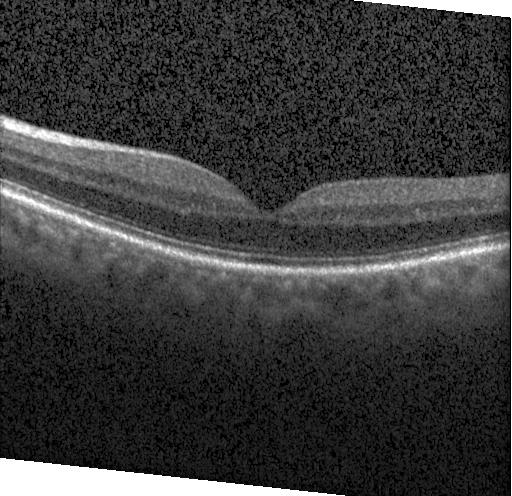
OCT line scan. Heidelberg Spectralis OCT system. Spectral-domain optical coherence tomography. Horizontal scan through the fovea
Finding: no evidence of CNV, DME, or drusen.